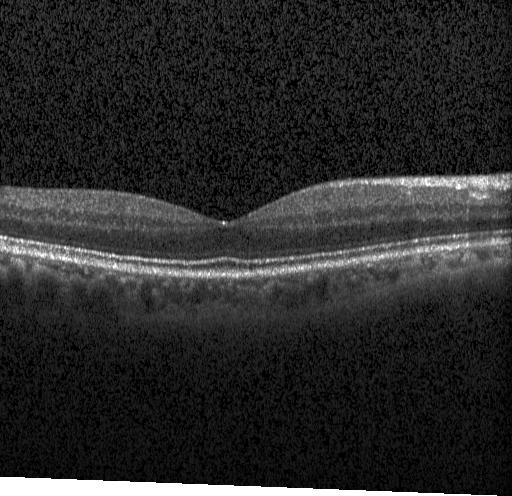 Optical coherence tomography B-scan
No choroidal neovascularization, diabetic macular edema, or drusen.